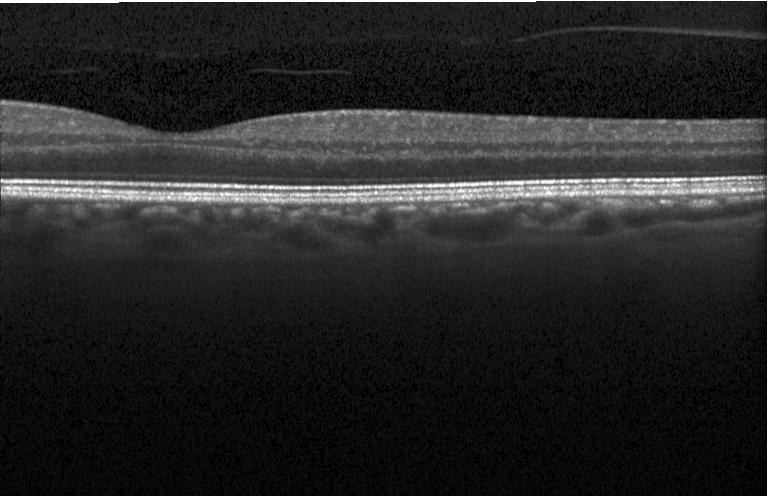

Assessment: neither choroidal neovascularization, diabetic macular edema, nor drusen.